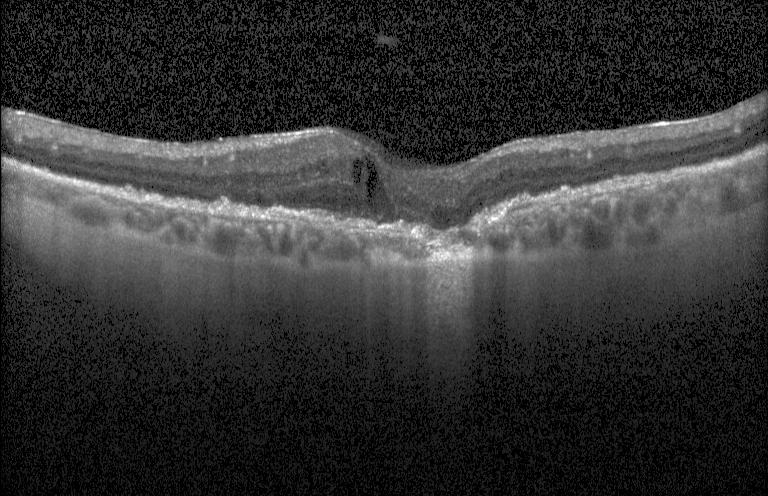

OCT B-scan — Assessment: choroidal neovascularization.